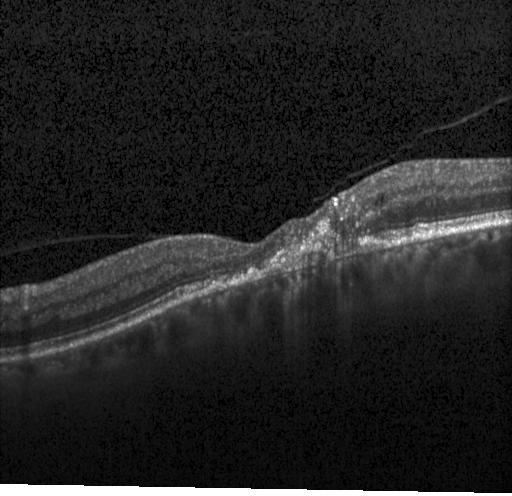
OCT finding: a choroidal neovascular membrane.